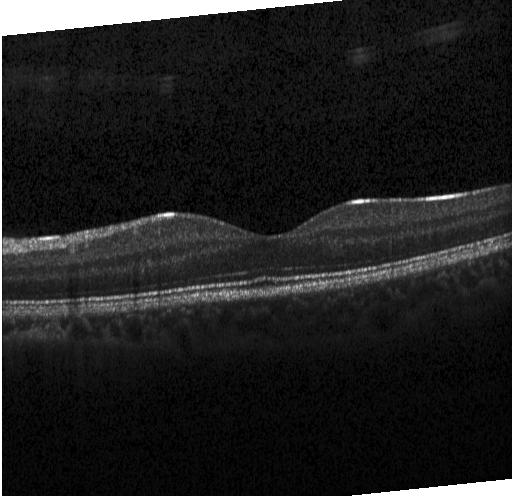

No choroidal neovascularization, no diabetic macular edema, and no drusen.